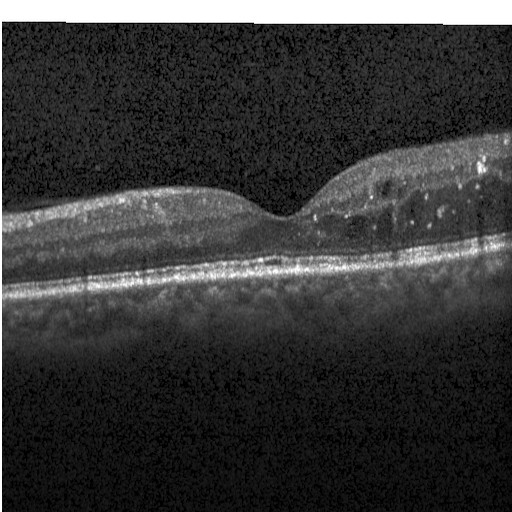
Fovea-centered, spectral-domain optical coherence tomography, acquired on a Heidelberg Spectralis, optical coherence tomography scan
Finding: diabetic macular edema.